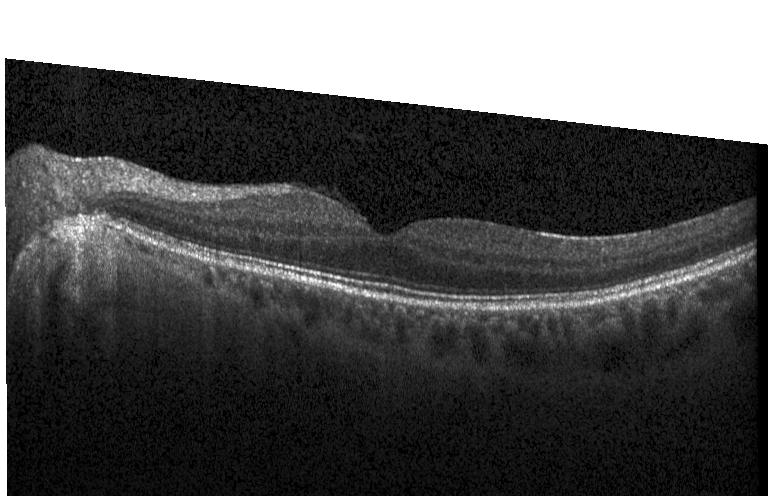

Impression: no evidence of choroidal neovascularization, diabetic macular edema, or drusen.